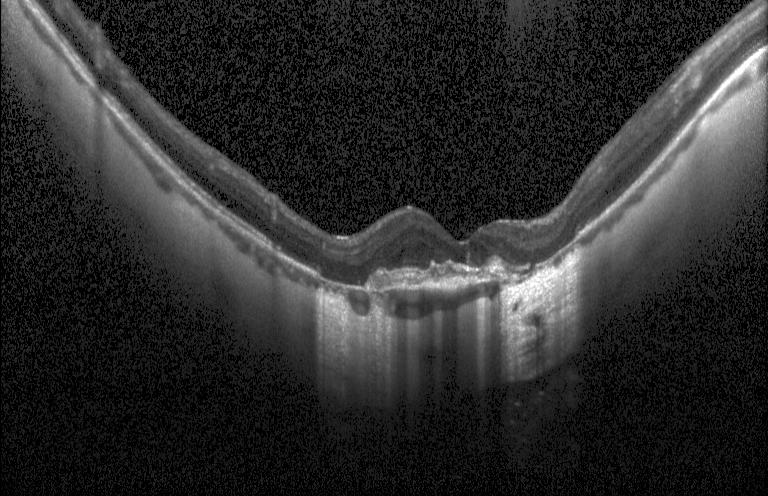

OCT B-scan.
The scan shows choroidal neovascularization (CNV).